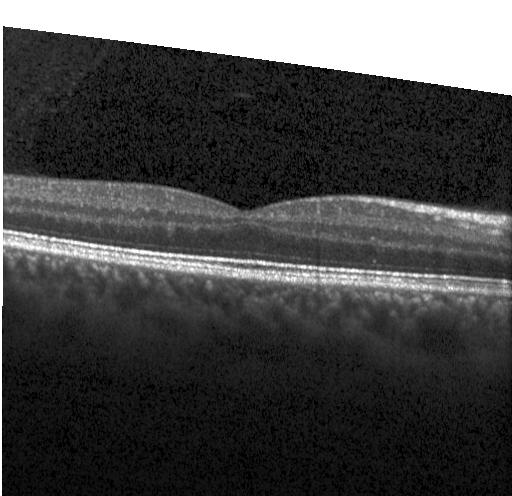 OCT line scan; acquired on a Heidelberg Spectralis — No choroidal neovascularization, no diabetic macular edema, and no drusen.